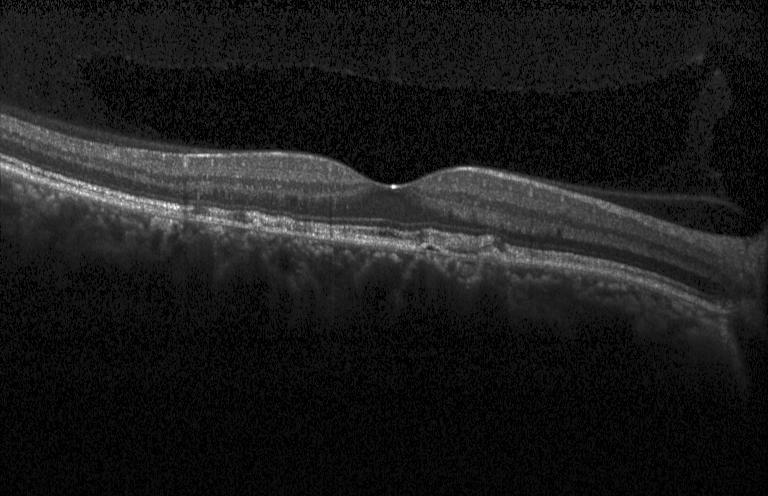 Macular scan; optical coherence tomography scan
Diagnosis: drusen.